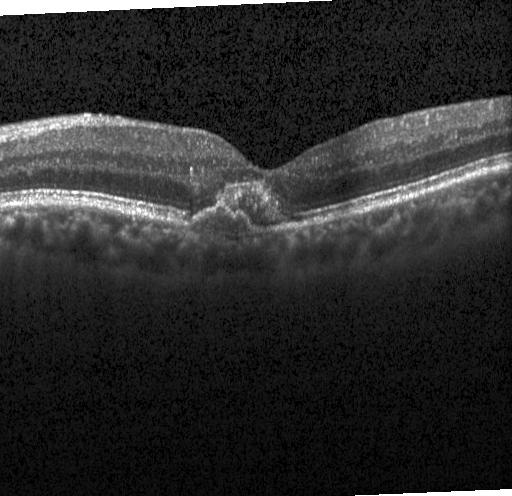
The scan shows a choroidal neovascular membrane.